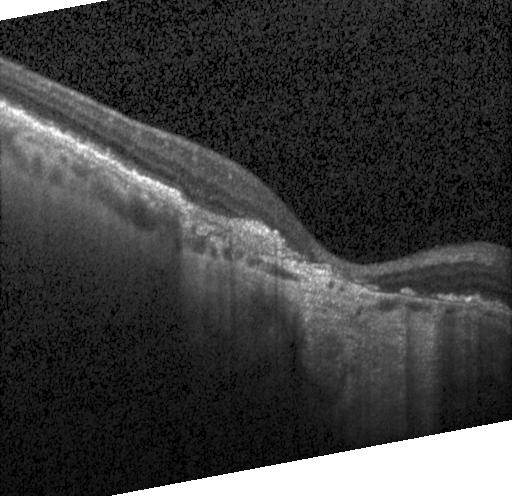
Spectral-domain optical coherence tomography, horizontal scan through the fovea, optical coherence tomography B-scan — OCT finding: choroidal neovascularization.